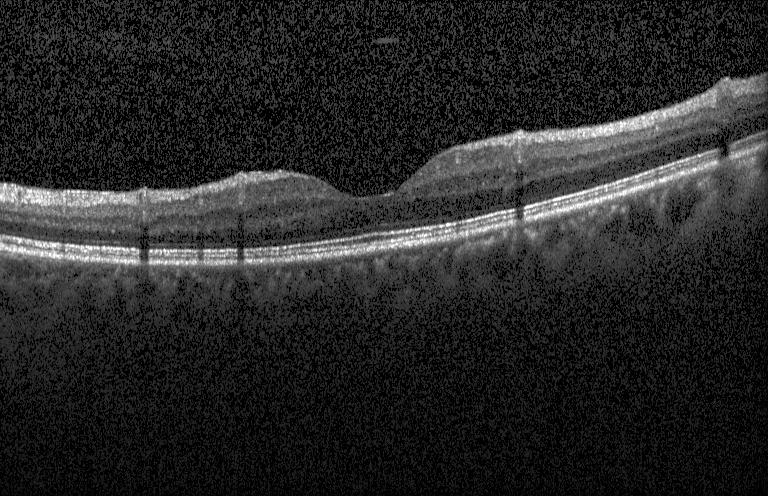

Assessment: neither choroidal neovascularization, diabetic macular edema, nor drusen.